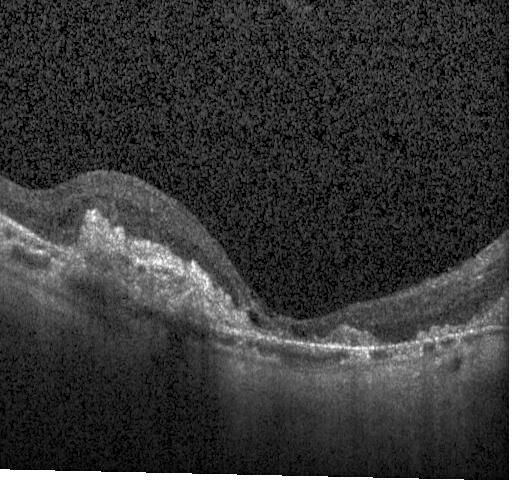
SD-OCT · acquired on a Heidelberg Spectralis · optical coherence tomography B-scan — Choroidal neovascularization (CNV).